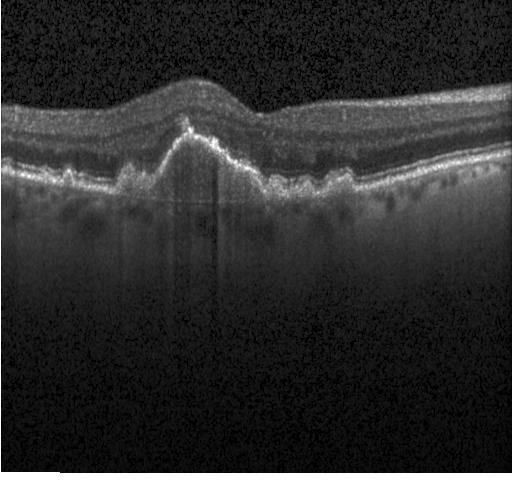
Acquired on a Heidelberg Spectralis · optical coherence tomography scan — Macular OCT: choroidal neovascularization.